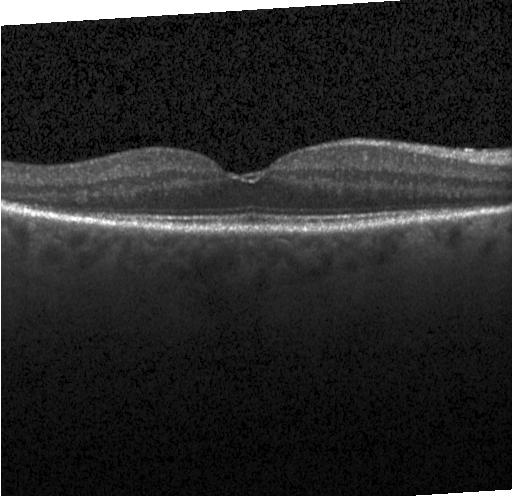

Dx: no CNV, DME, or drusen.